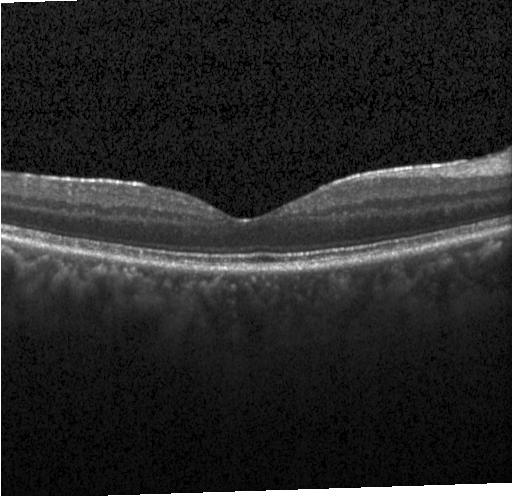 No evidence of choroidal neovascularization, diabetic macular edema, or drusen.